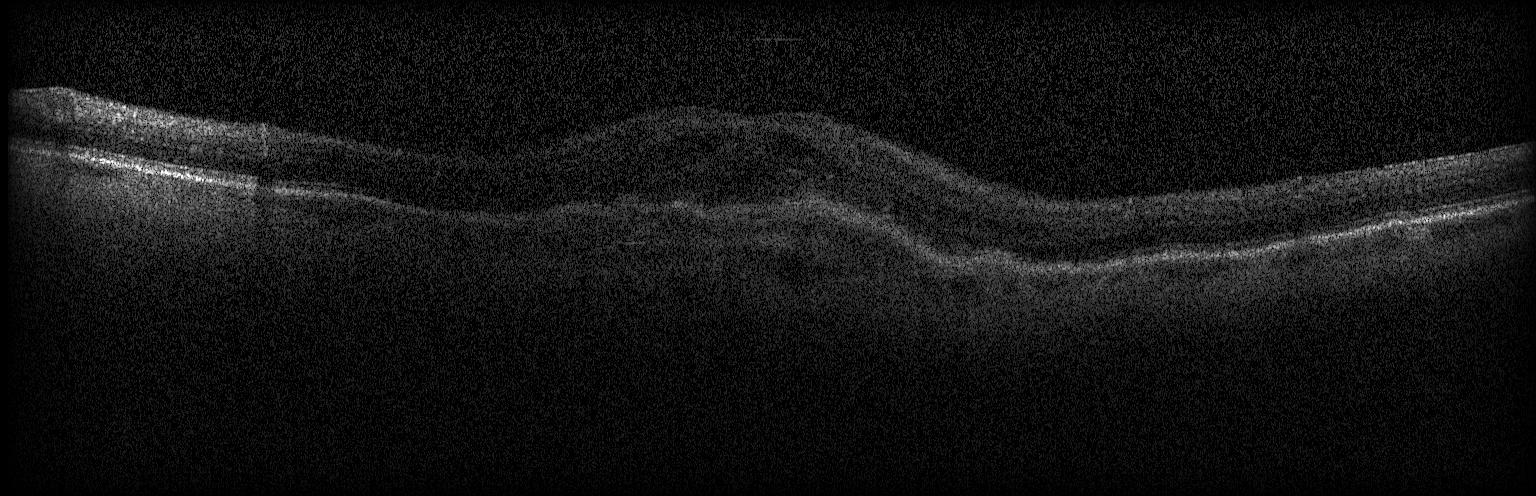

Fovea-centered, optical coherence tomography B-scan — Dx: CNV.